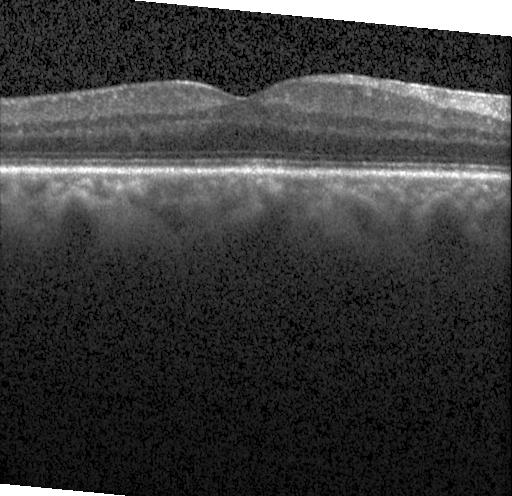 Retinal OCT cross-section
The scan shows neither CNV, DME, nor drusen.